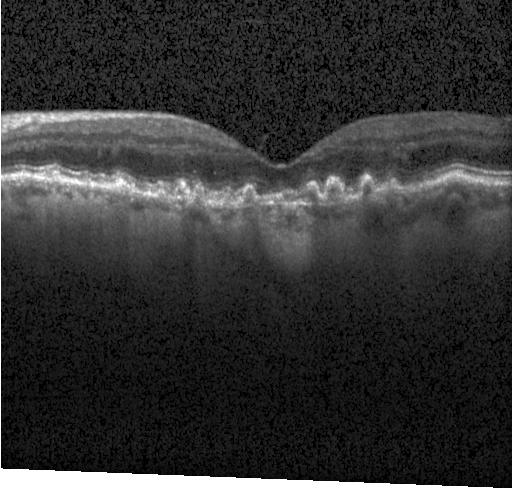

Centered on the fovea · OCT line scan · spectral-domain OCT · Heidelberg Spectralis OCT system.
Finding: multiple drusen.